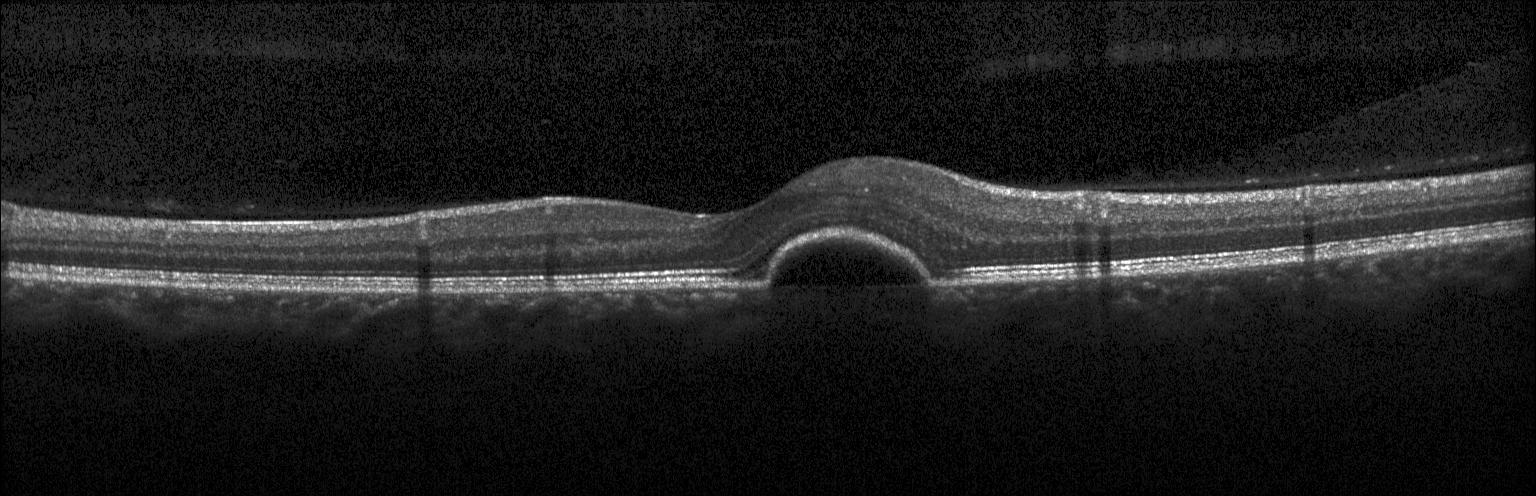

Optical coherence tomography B-scan, spectral-domain OCT, centered on the fovea
A choroidal neovascular membrane.